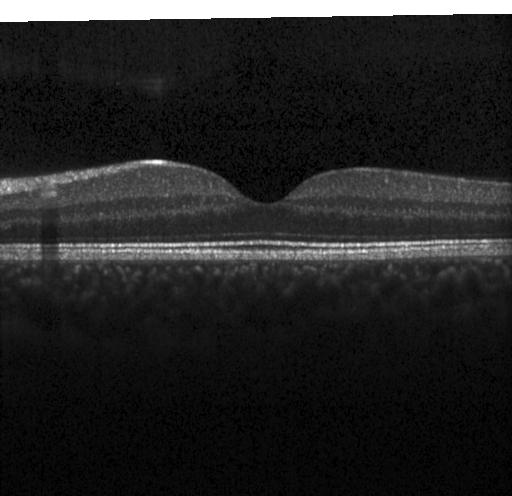

OCT line scan.
Diagnosis: no choroidal neovascularization, no diabetic macular edema, and no drusen.